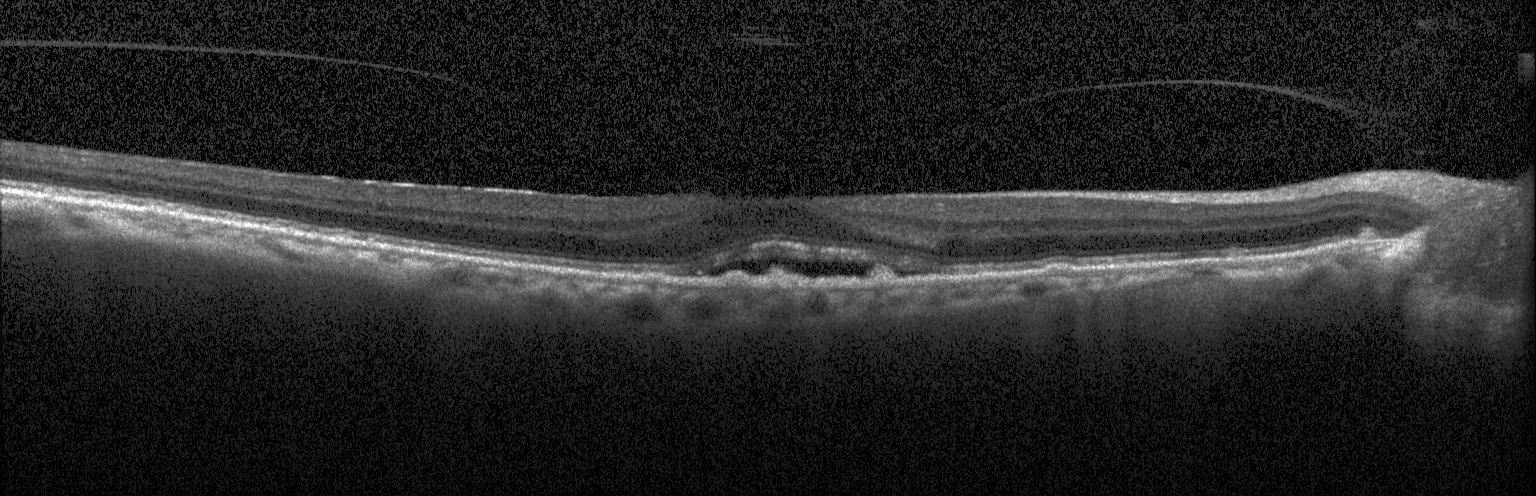
Fovea-centered · Heidelberg Spectralis · SD-OCT · retinal OCT B-scan. Finding: a choroidal neovascular membrane.